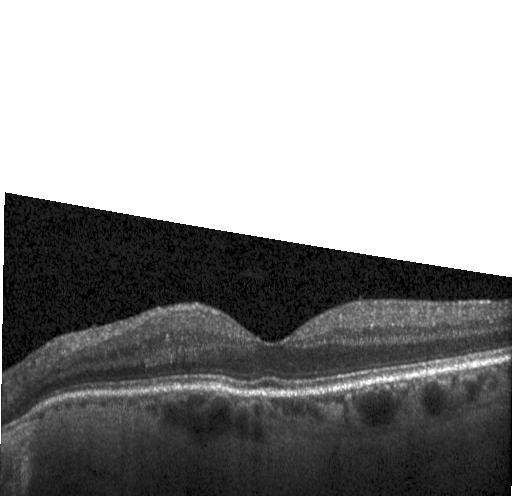

OCT B-scan showing no evidence of choroidal neovascularization, diabetic macular edema, or drusen.